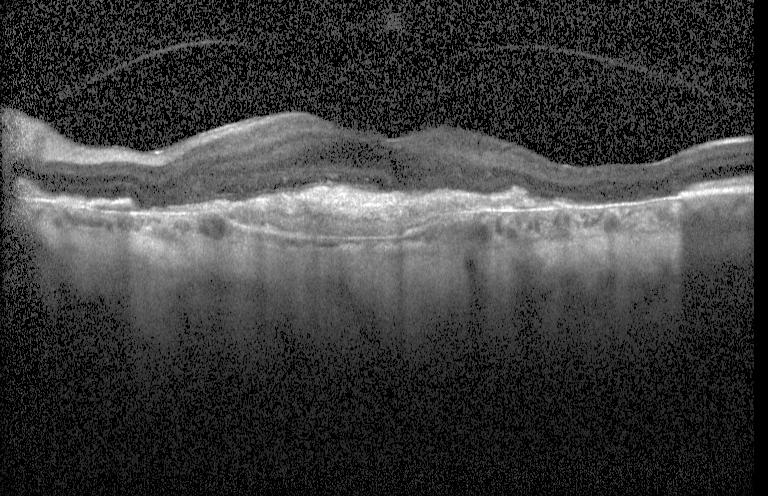
Retinal OCT cross-section. Assessment: choroidal neovascularization (CNV).